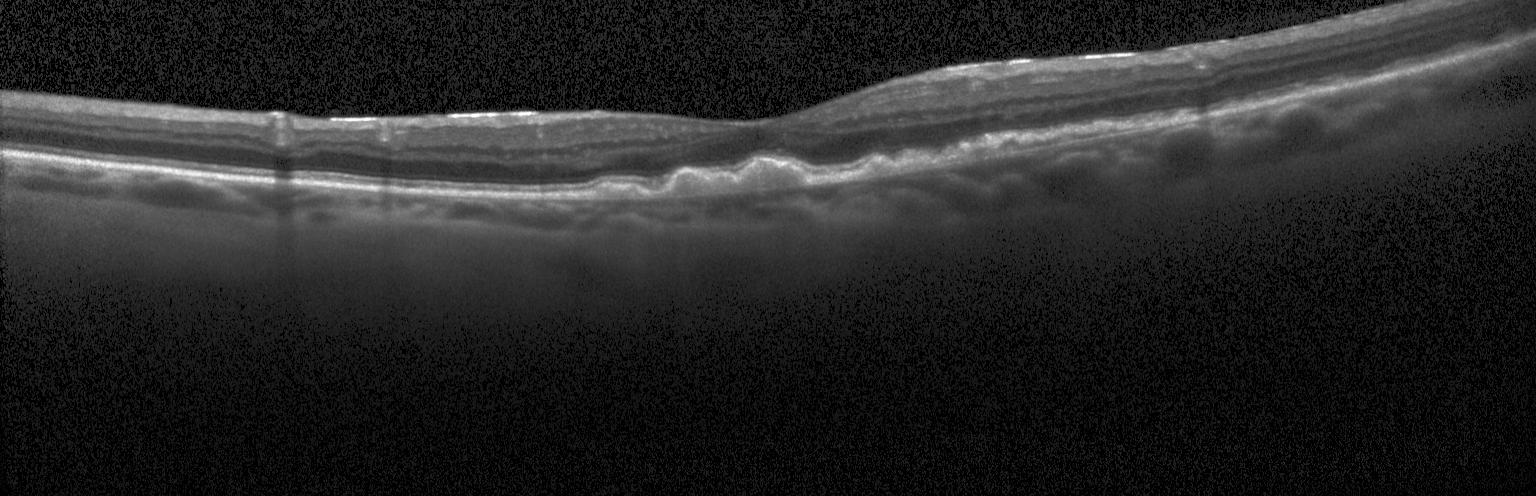

Retinal OCT cross-section. Drusen.